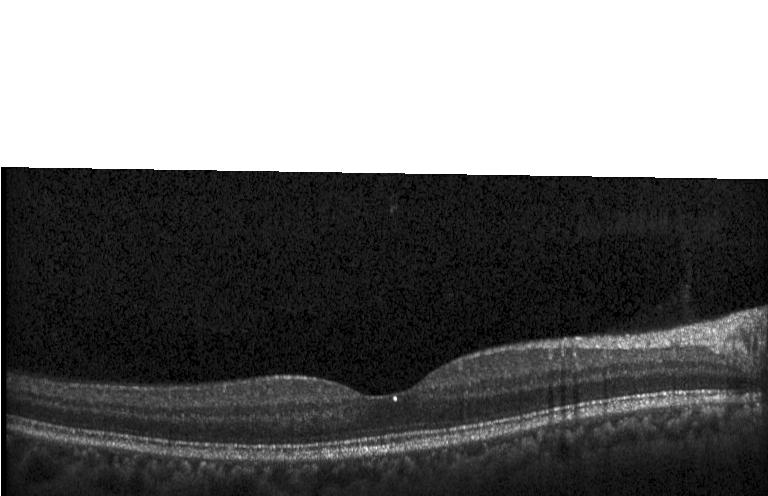

Impression: no evidence of CNV, DME, or drusen.